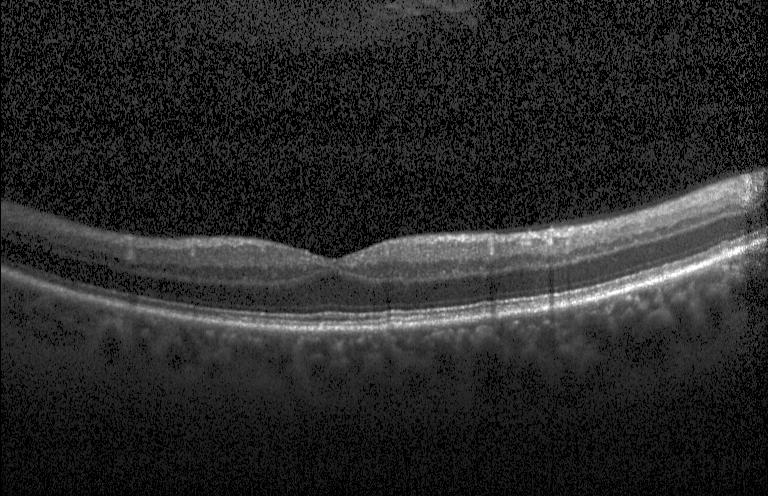
Retinal OCT cross-section · Heidelberg Spectralis · spectral-domain OCT.
Assessment: no choroidal neovascularization, diabetic macular edema, or drusen.